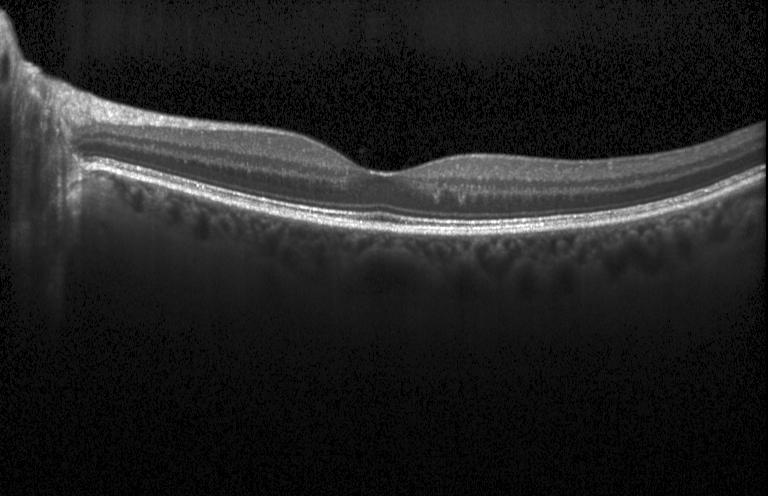

OCT line scan — Dx: no choroidal neovascularization, diabetic macular edema, or drusen.